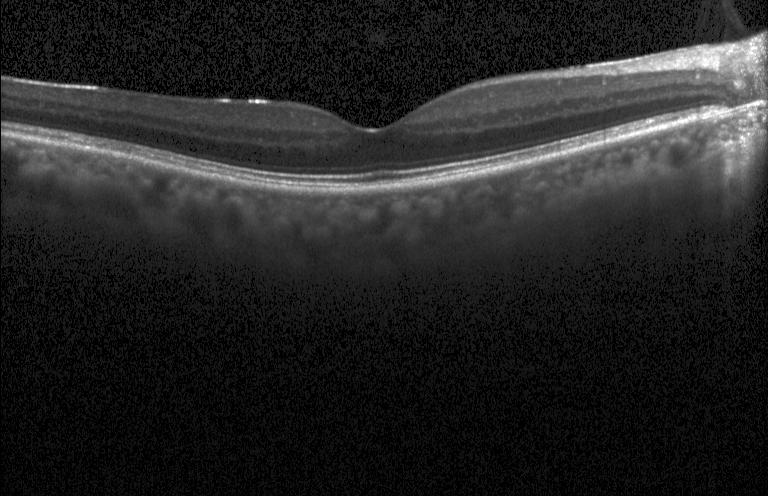

Optical coherence tomography B-scan; fovea-centered — Impression: no CNV, no DME, and no drusen.